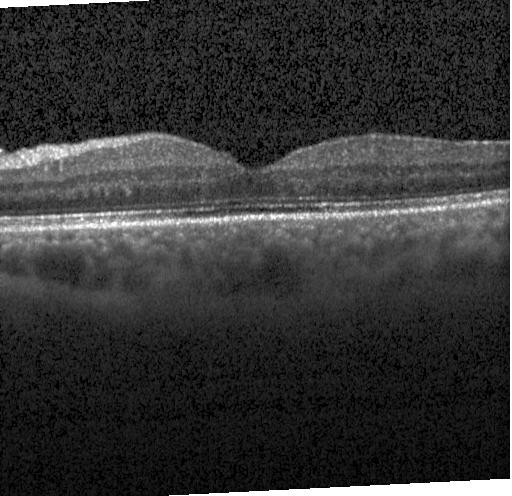

OCT scan showing no choroidal neovascularization, diabetic macular edema, or drusen.